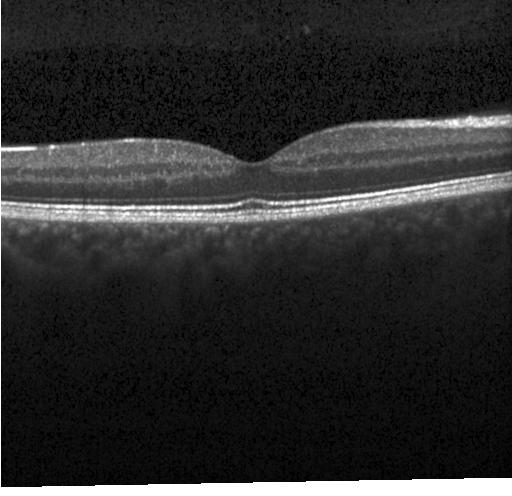

Macular OCT demonstrating neither choroidal neovascularization, diabetic macular edema, nor drusen.